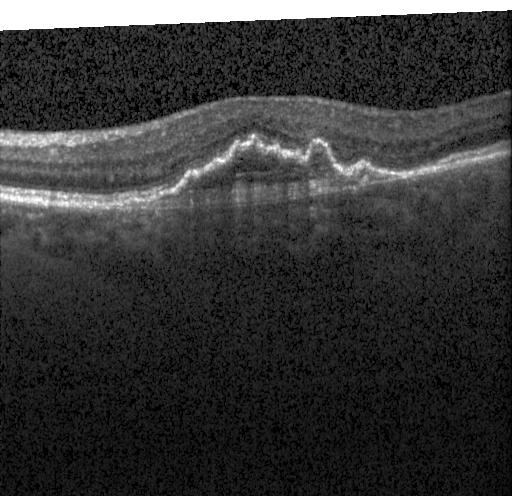

Retinal OCT B-scan. Impression: choroidal neovascularization.